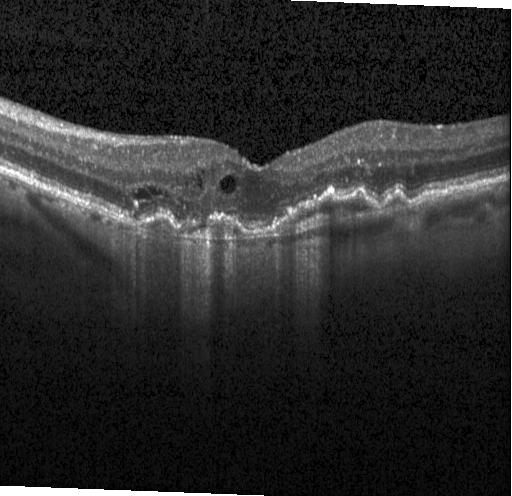 Spectral-domain OCT B-scan: choroidal neovascularization (CNV).